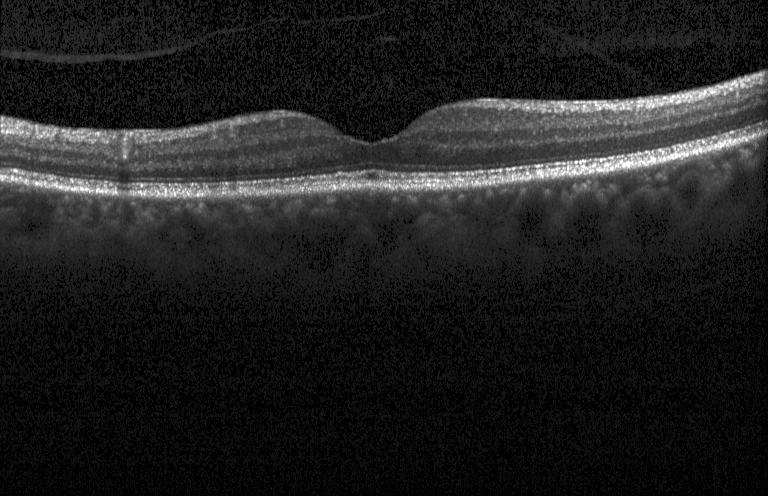

Optical coherence tomography scan. Diagnosis: no choroidal neovascularization, no diabetic macular edema, and no drusen.